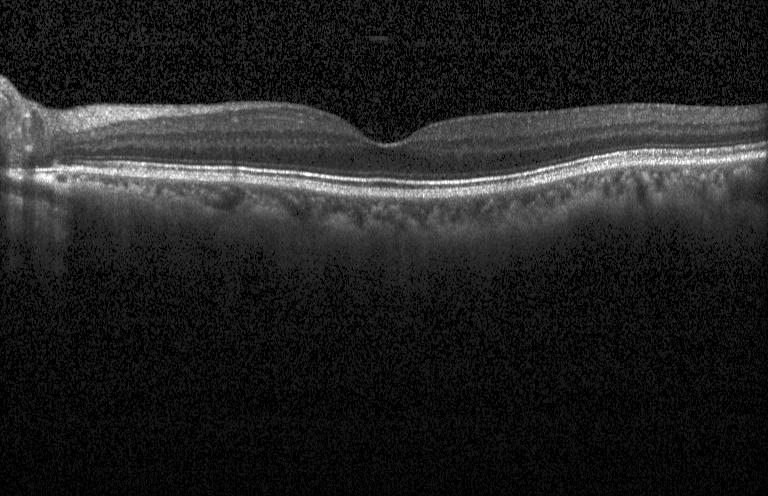
Heidelberg Spectralis; horizontal scan through the fovea; optical coherence tomography B-scan.
This B-scan demonstrates no choroidal neovascularization, no diabetic macular edema, and no drusen.